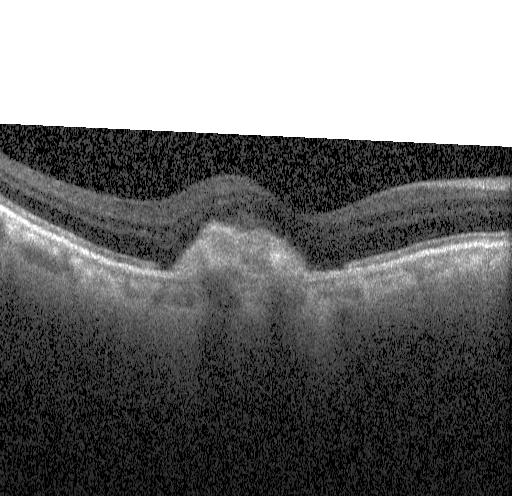
Retinal OCT B-scan. SD-OCT. Horizontal scan through the fovea.
Assessment: choroidal neovascularization.